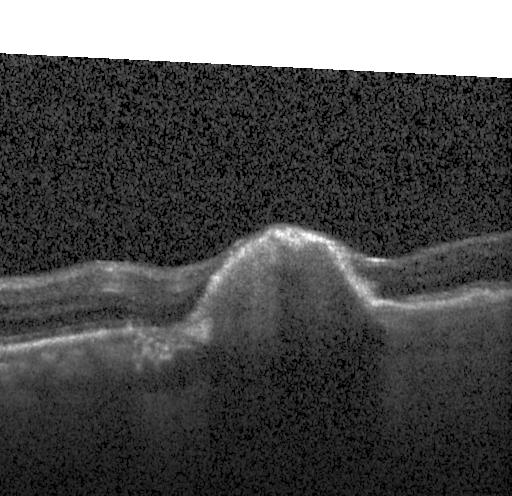 Macular OCT demonstrating CNV.